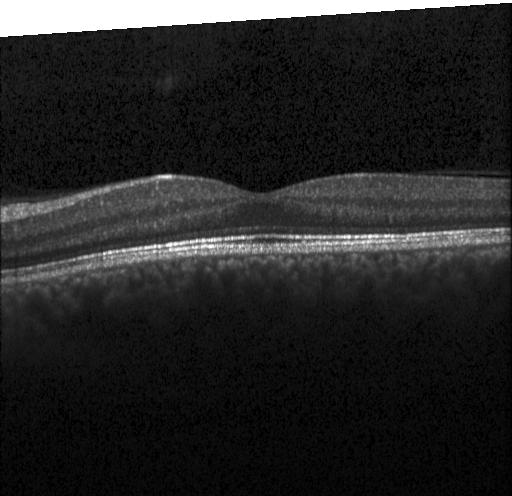
Retinal OCT B-scan. Finding: no choroidal neovascularization, no diabetic macular edema, and no drusen.